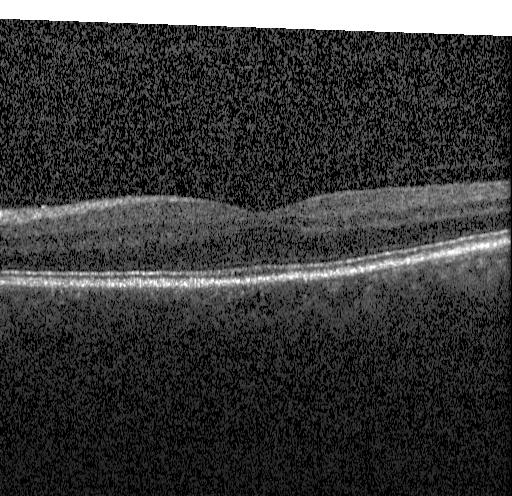
Heidelberg Spectralis; SD-OCT; optical coherence tomography B-scan; horizontal scan through the fovea — Finding: no choroidal neovascularization, no diabetic macular edema, and no drusen.